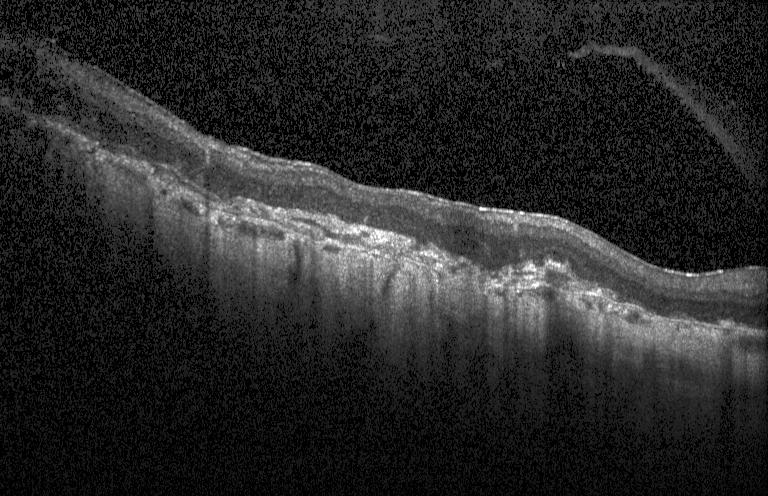
Spectral-domain OCT B-scan: choroidal neovascularization (CNV).